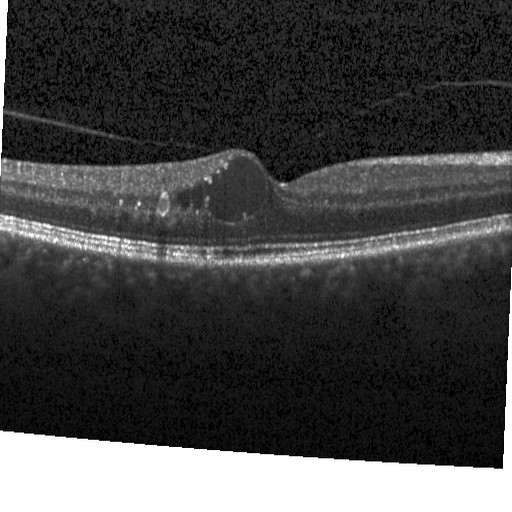

Assessment: DME.